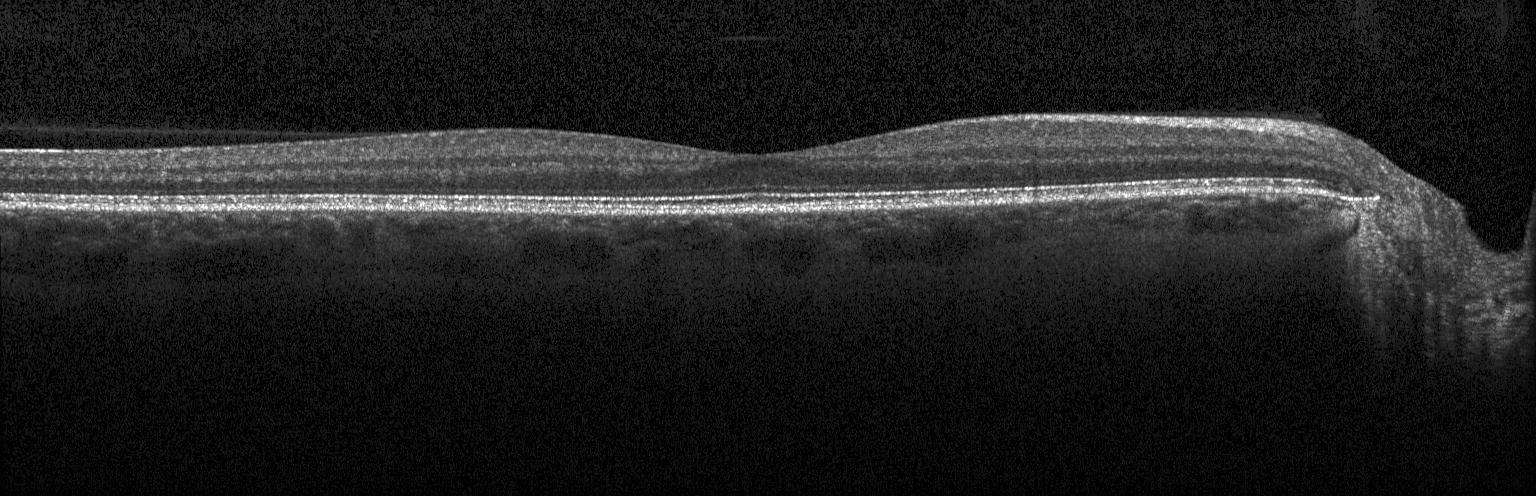

The scan shows no choroidal neovascularization, no diabetic macular edema, and no drusen.